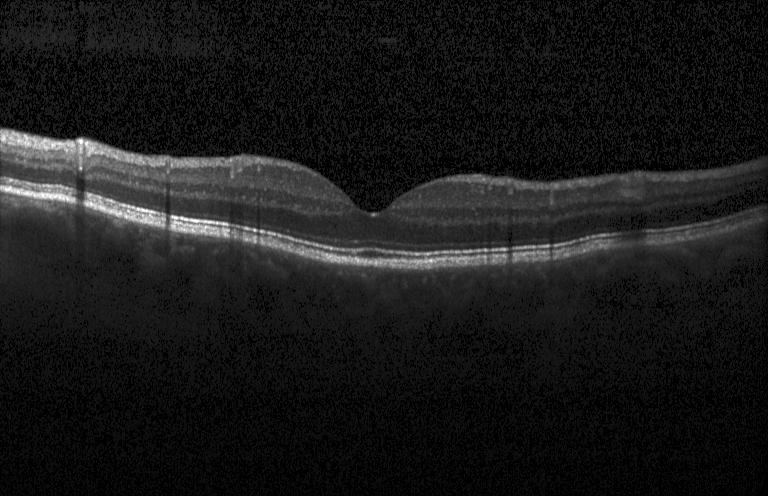 OCT scan showing no choroidal neovascularization, no diabetic macular edema, and no drusen.